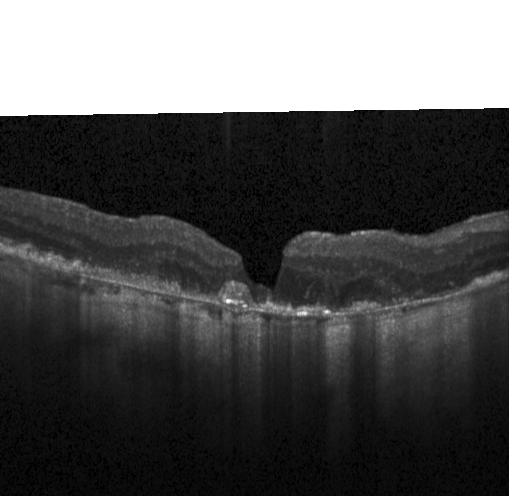
This B-scan demonstrates a choroidal neovascular membrane.